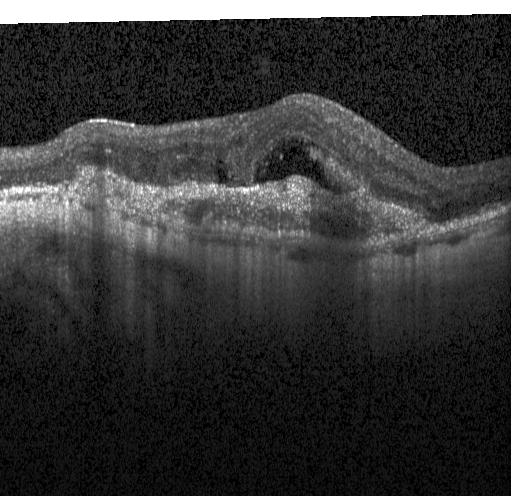

Through the macula. Acquired on a Heidelberg Spectralis. Retinal OCT B-scan. Spectral-domain OCT
Impression: choroidal neovascularization (CNV).